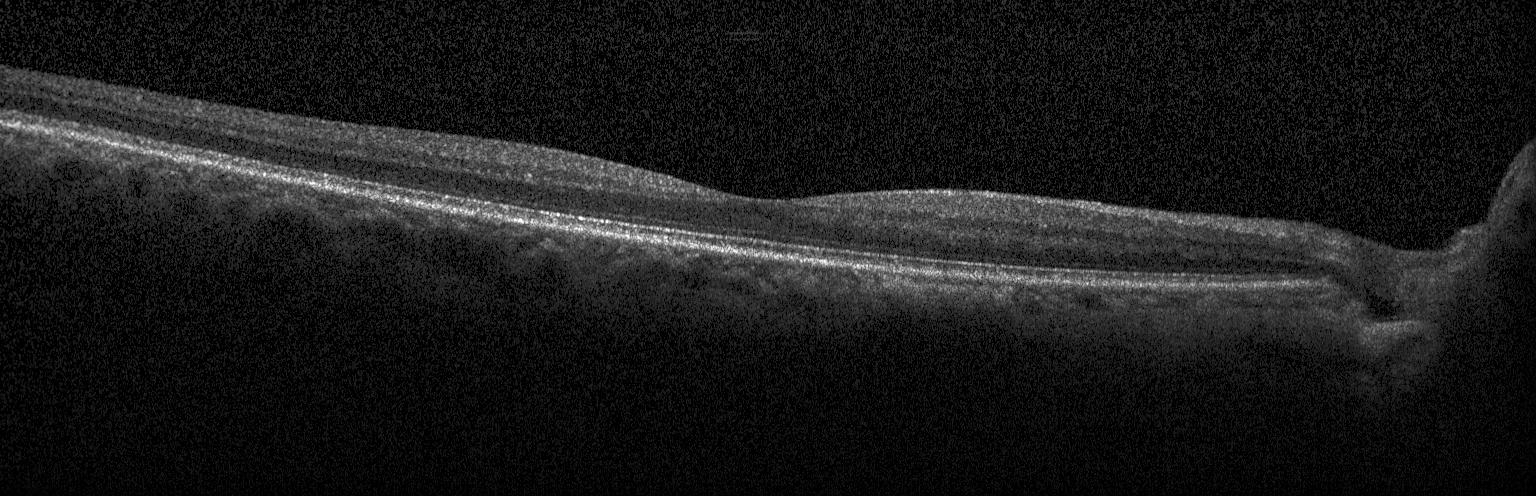

Impression: no evidence of choroidal neovascularization, diabetic macular edema, or drusen.